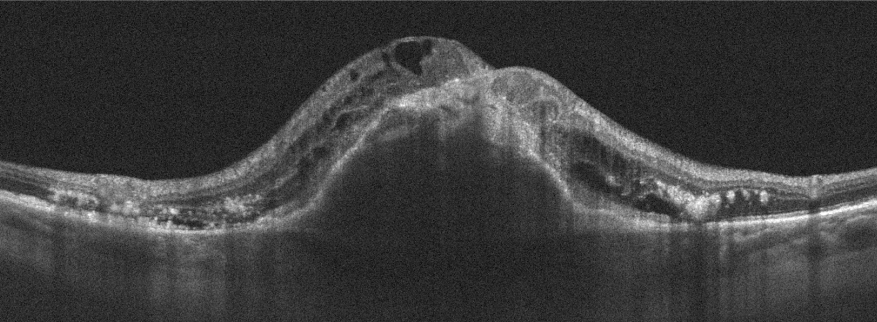
Retinal OCT cross-section
Impression: AMD.